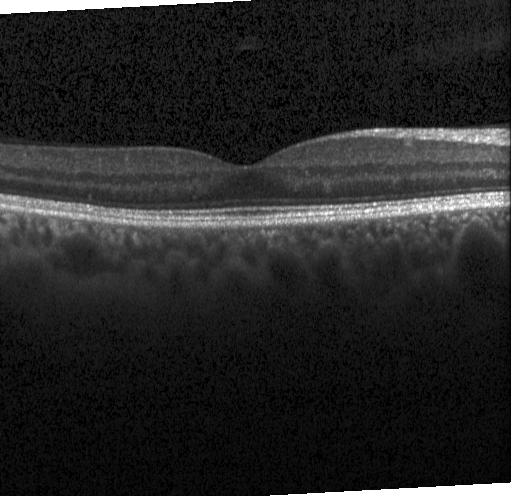

Optical coherence tomography B-scan · acquired on a Heidelberg Spectralis · SD-OCT · fovea-centered — This B-scan demonstrates neither CNV, DME, nor drusen.